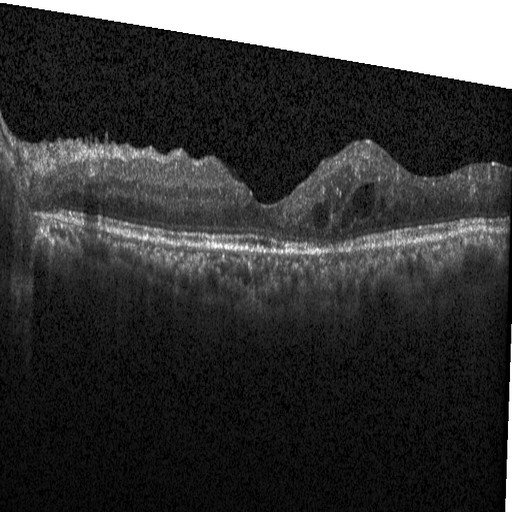
Optical coherence tomography scan, macular scan, Heidelberg Spectralis OCT system. This B-scan demonstrates diabetic macular edema (DME).